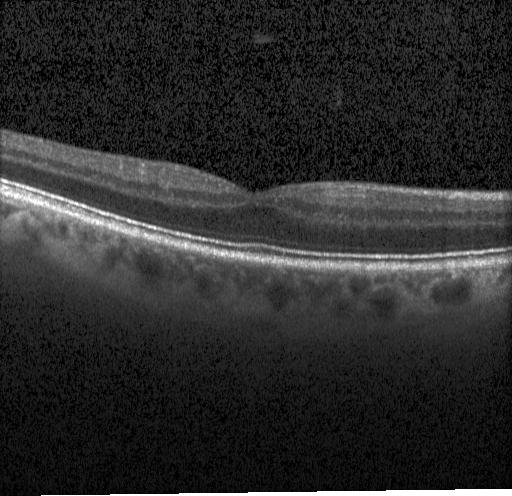

OCT line scan. Diagnosis: no evidence of choroidal neovascularization, diabetic macular edema, or drusen.